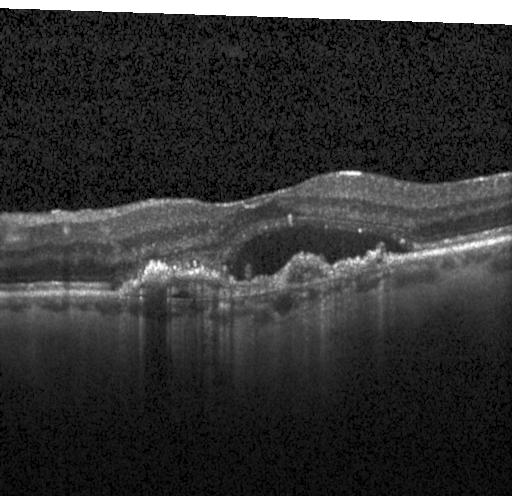

OCT line scan — Macular OCT: a choroidal neovascular membrane.